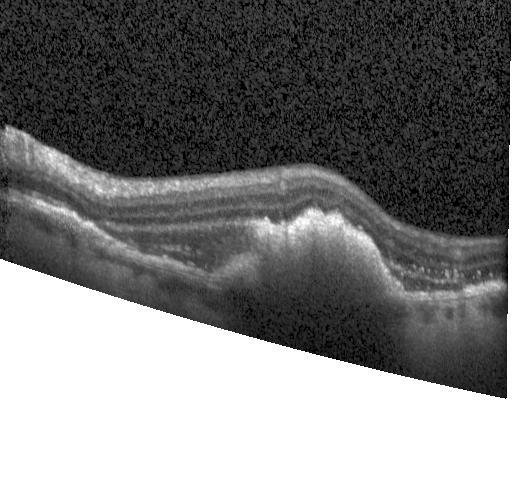

OCT B-scan. This B-scan demonstrates CNV.